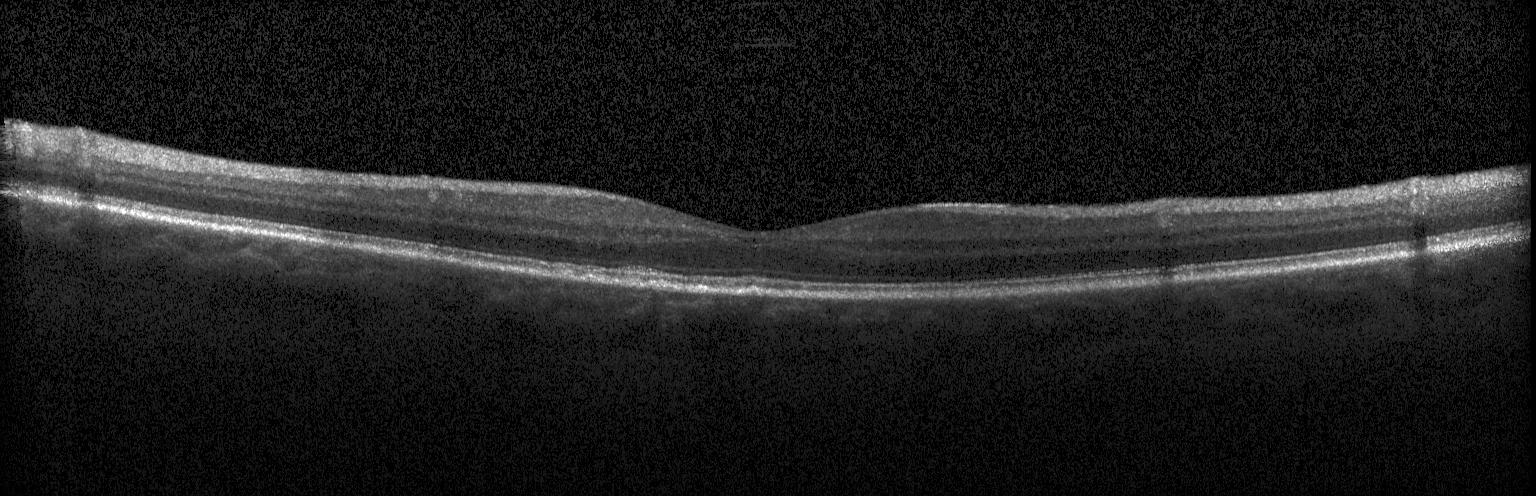
Acquired on a Heidelberg Spectralis. Optical coherence tomography scan. SD-OCT
Impression: no CNV, DME, or drusen.